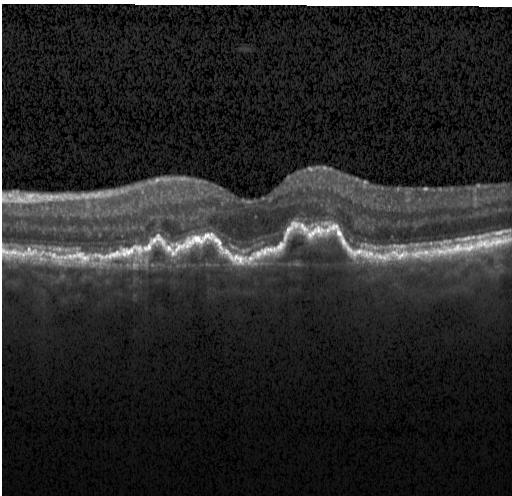 Optical coherence tomography scan · instrument: Heidelberg Spectralis. Diagnosis: CNV.